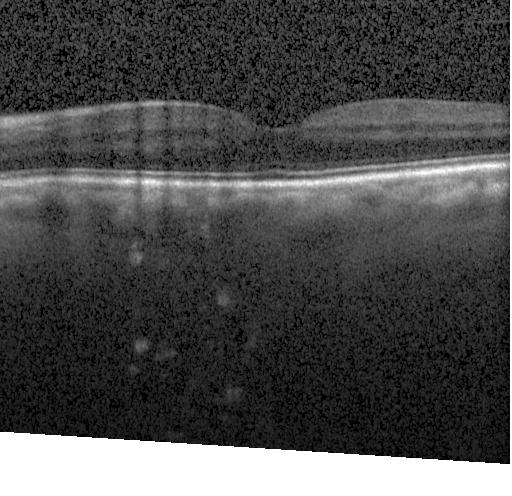
Retinal OCT cross-section, spectral-domain OCT, horizontal scan through the fovea — The scan shows neither CNV, DME, nor drusen.